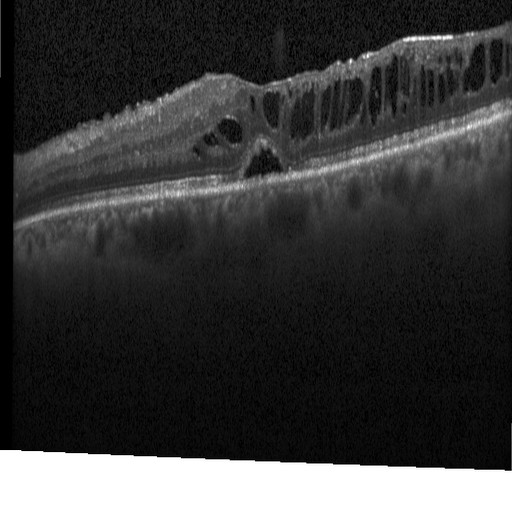 Retinal OCT cross-section showing DME.